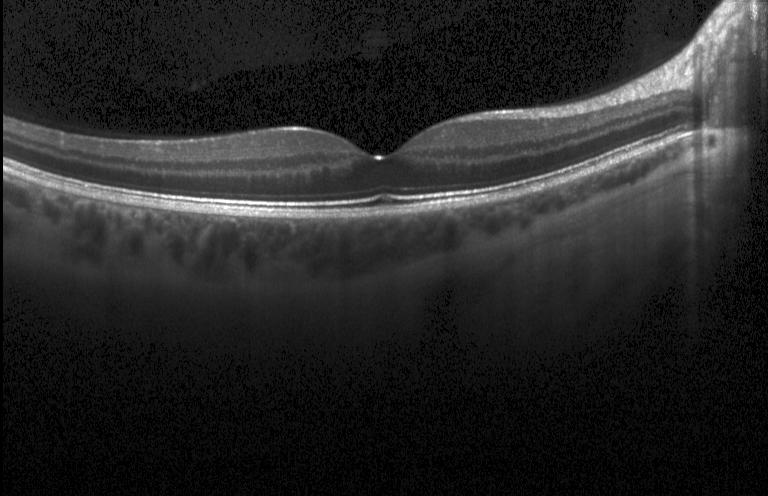
Macular scan, Heidelberg Spectralis OCT system, OCT line scan
The scan shows no evidence of choroidal neovascularization, diabetic macular edema, or drusen.